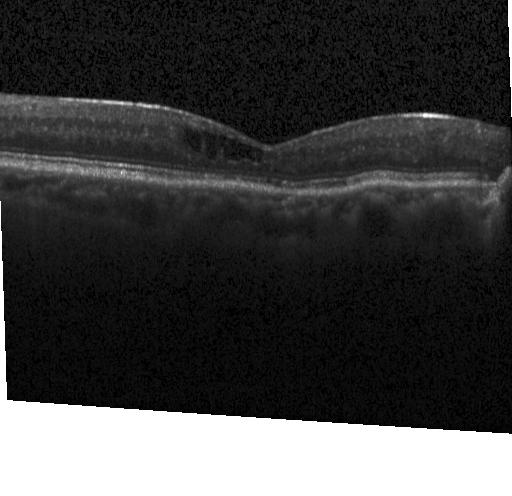 Retinal OCT B-scan; horizontal scan through the fovea. Diagnosis: DME.